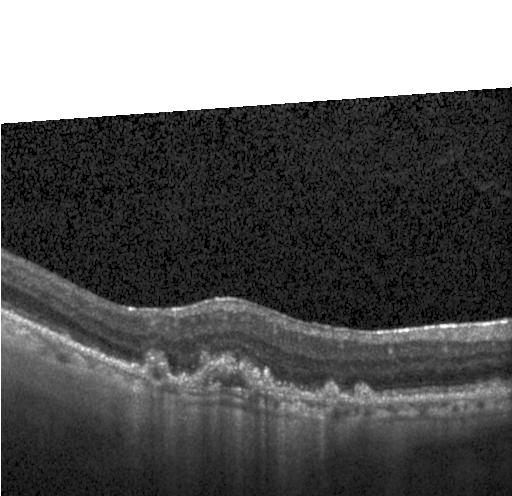
Instrument: Heidelberg Spectralis, optical coherence tomography B-scan. Diagnosis: CNV.